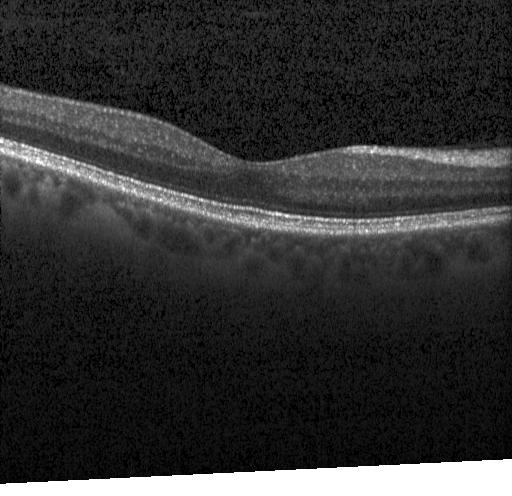 Spectral-domain OCT B-scan: no evidence of choroidal neovascularization, diabetic macular edema, or drusen.